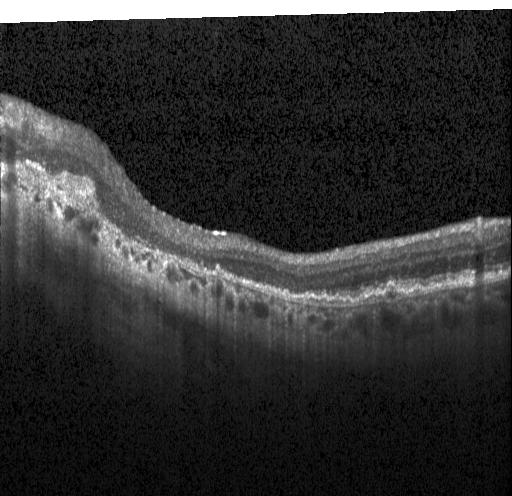

Through the macula, retinal OCT B-scan, SD-OCT, acquired on a Heidelberg Spectralis.
OCT finding: a choroidal neovascular membrane.